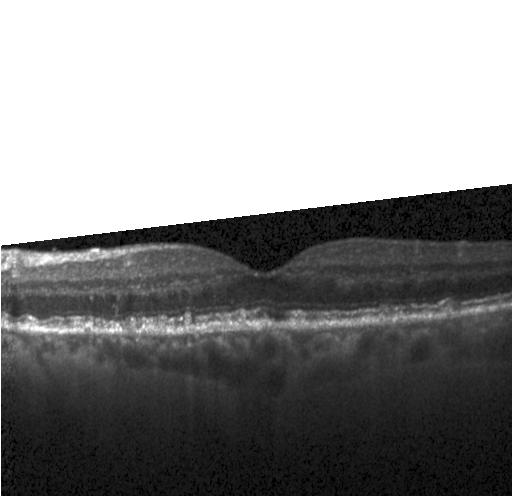
Retinal OCT cross-section; instrument: Heidelberg Spectralis — Impression: sub-RPE drusenoid deposits.